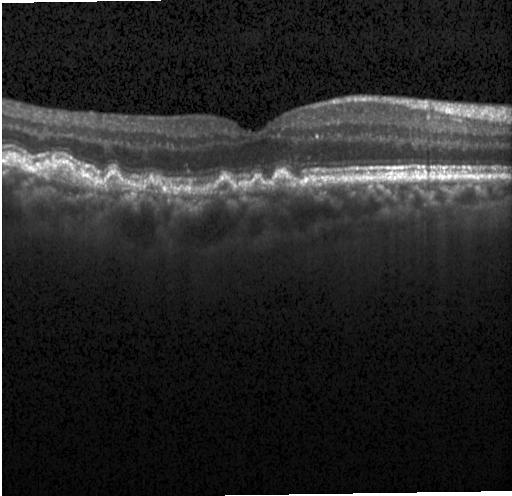 This B-scan demonstrates sub-RPE drusenoid deposits.